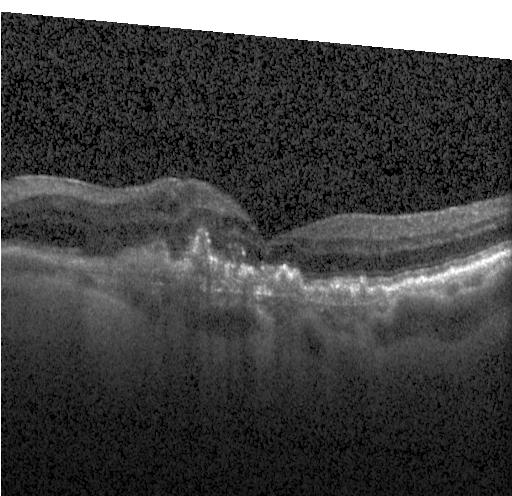 Through the macula; acquired on a Heidelberg Spectralis; optical coherence tomography B-scan; spectral-domain OCT — Diagnosis: a choroidal neovascular membrane.